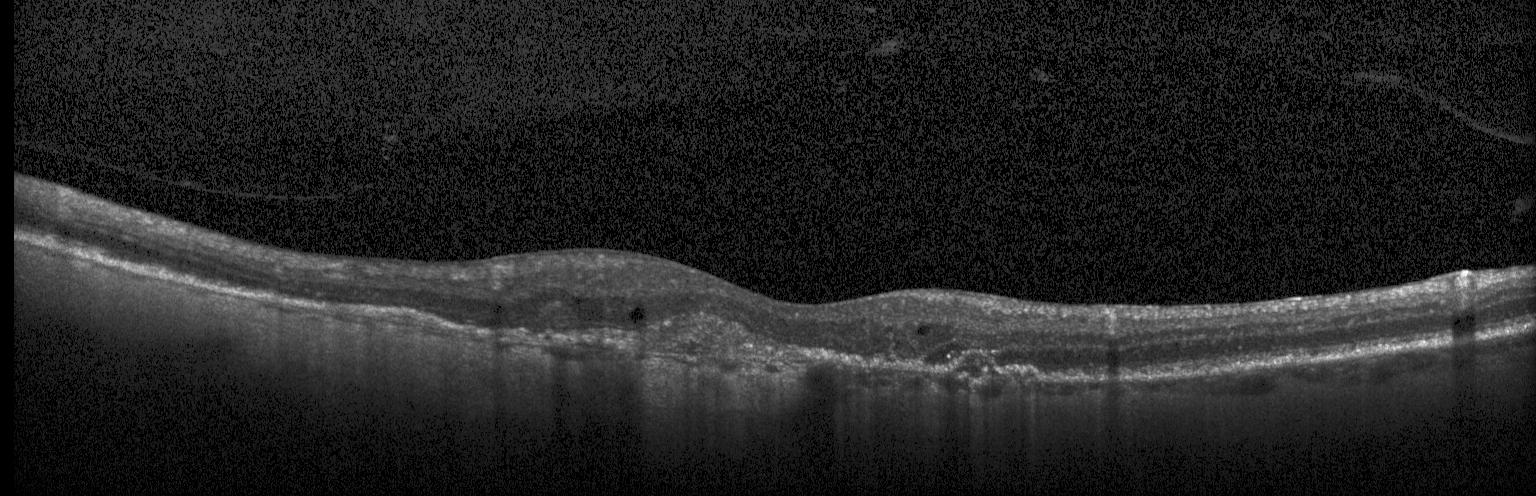

OCT line scan. Acquired on a Heidelberg Spectralis.
Assessment: choroidal neovascularization (CNV).